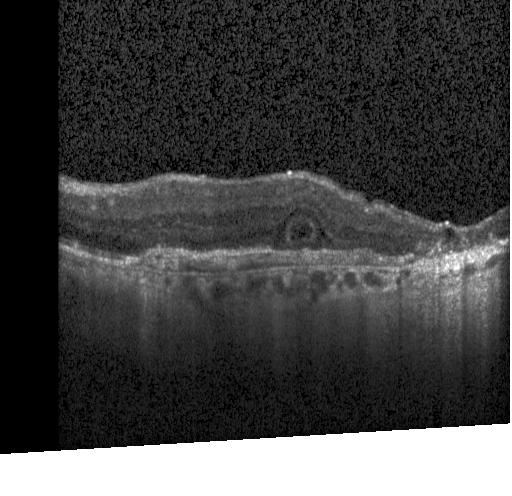

Spectral-domain optical coherence tomography. Acquired on a Heidelberg Spectralis. OCT line scan. Fovea-centered.
Choroidal neovascularization (CNV).